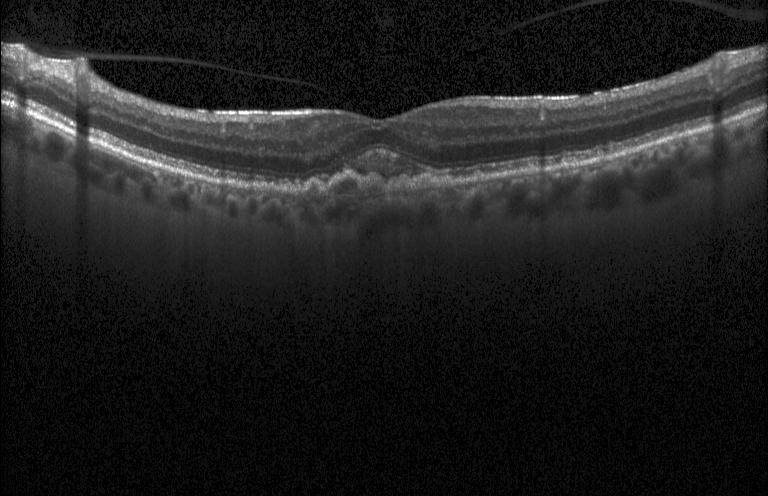
Spectral-domain OCT B-scan: choroidal neovascularization (CNV).